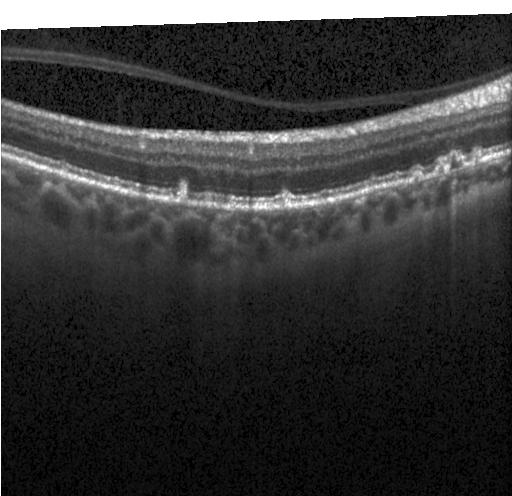

Heidelberg Spectralis OCT system. SD-OCT. Optical coherence tomography scan
Finding: drusen.